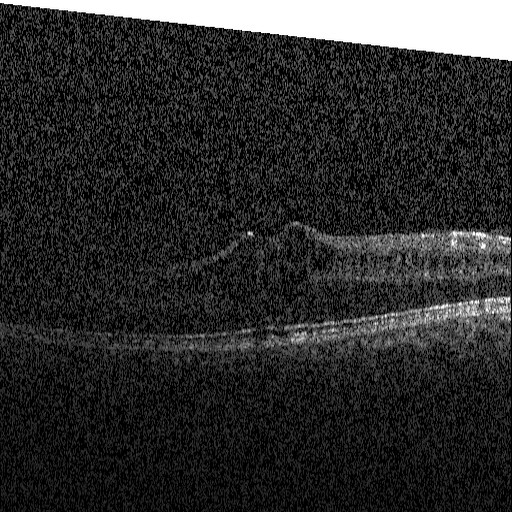

Heidelberg Spectralis · OCT B-scan.
The scan shows diabetic macular edema.